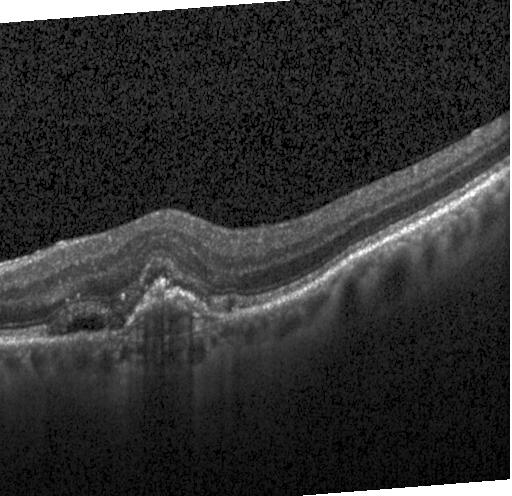 Retinal OCT cross-section
OCT finding: a choroidal neovascular membrane.